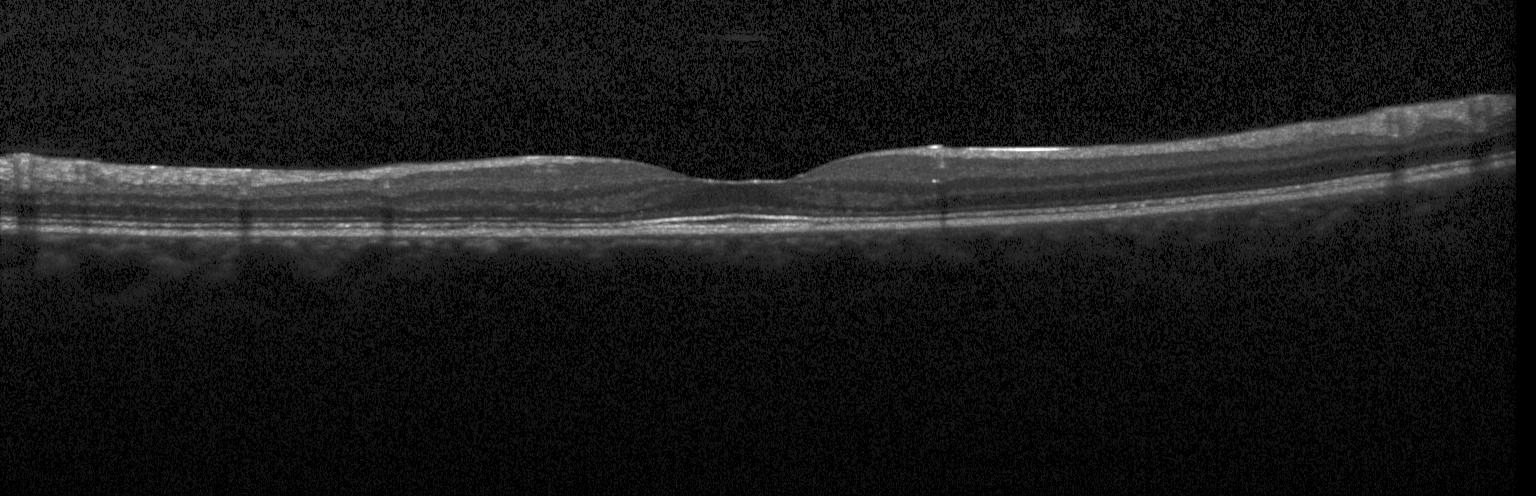

OCT finding: no choroidal neovascularization, diabetic macular edema, or drusen.